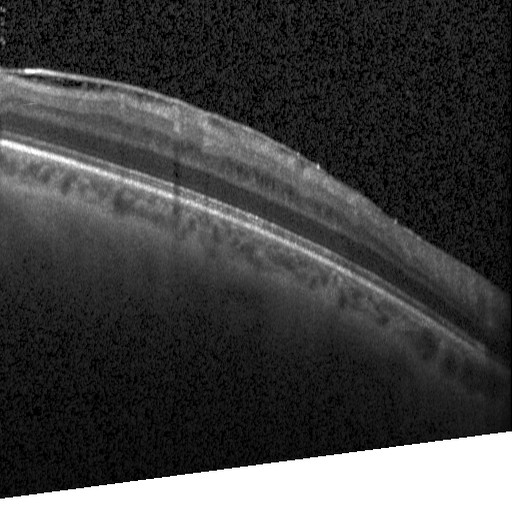
OCT finding: diabetic macular edema (DME).